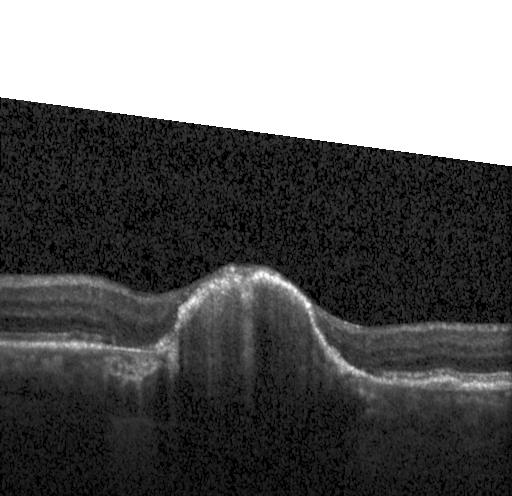 OCT B-scan.
Diagnosis: a choroidal neovascular membrane.